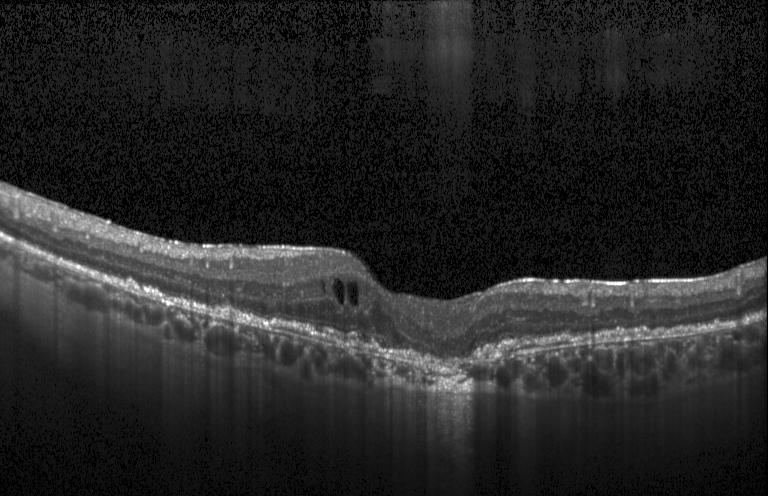 OCT B-scan. Diagnosis: a choroidal neovascular membrane.